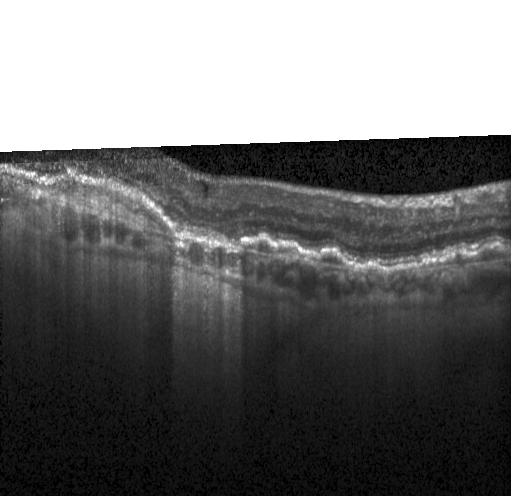

Finding: a choroidal neovascular membrane.